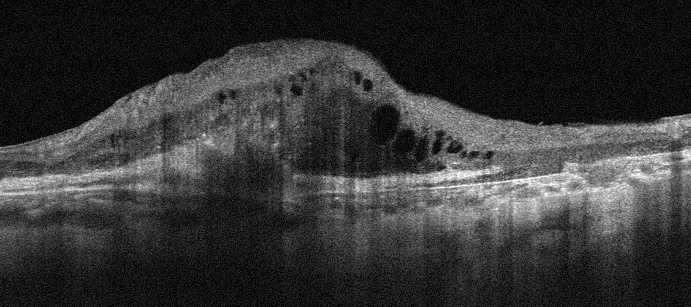 Macular scan, OCT B-scan.
Diagnosis: age-related macular degeneration.